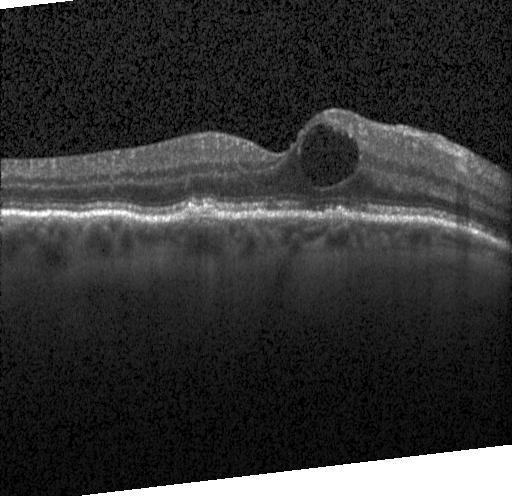

Macular OCT demonstrating CNV.